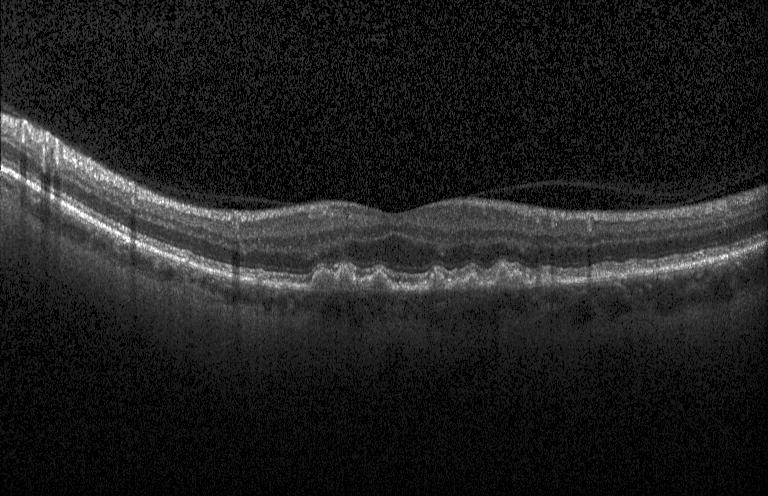

Retinal OCT cross-section · acquired on a Heidelberg Spectralis · spectral-domain OCT.
The scan shows sub-RPE drusenoid deposits.